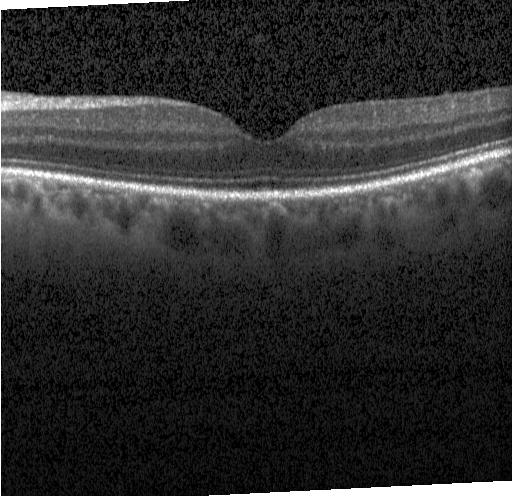 Retinal OCT cross-section; spectral-domain optical coherence tomography — This B-scan demonstrates no choroidal neovascularization, diabetic macular edema, or drusen.